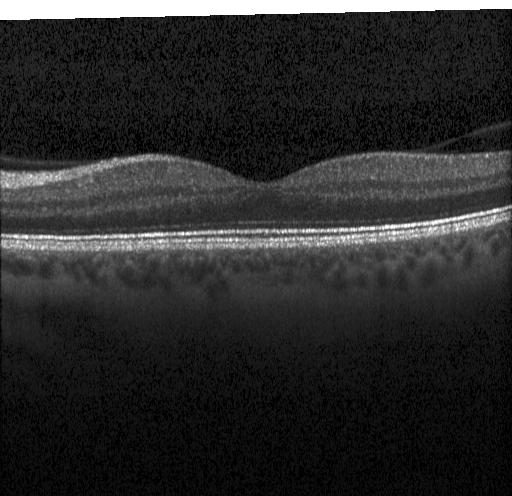
Spectral-domain optical coherence tomography, macular scan, OCT B-scan — OCT finding: no choroidal neovascularization, no diabetic macular edema, and no drusen.